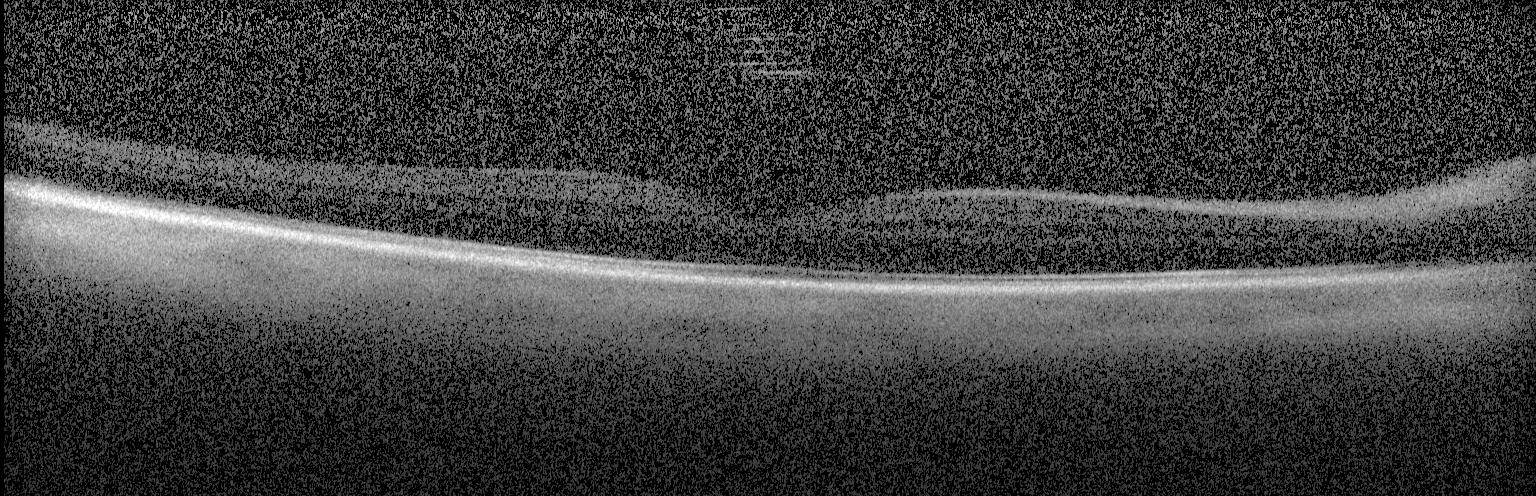 Retinal OCT B-scan, fovea-centered, Heidelberg Spectralis OCT system — Diagnosis: neither choroidal neovascularization, diabetic macular edema, nor drusen.